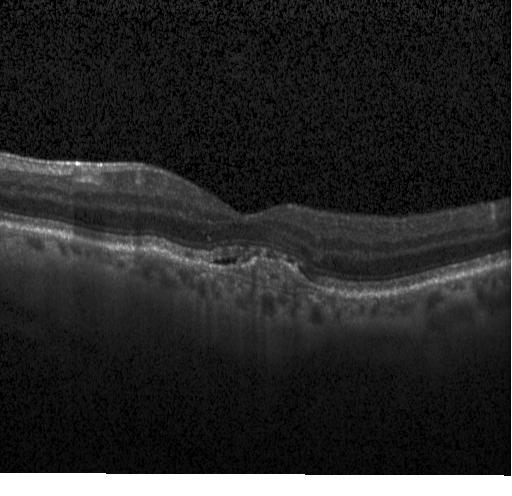

OCT finding: CNV.